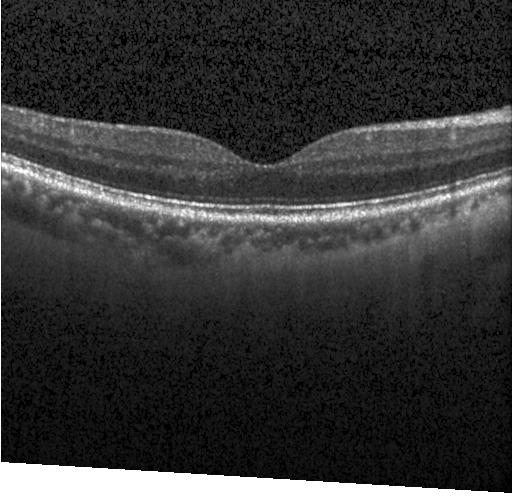 Heidelberg Spectralis; OCT B-scan — Neither choroidal neovascularization, diabetic macular edema, nor drusen.